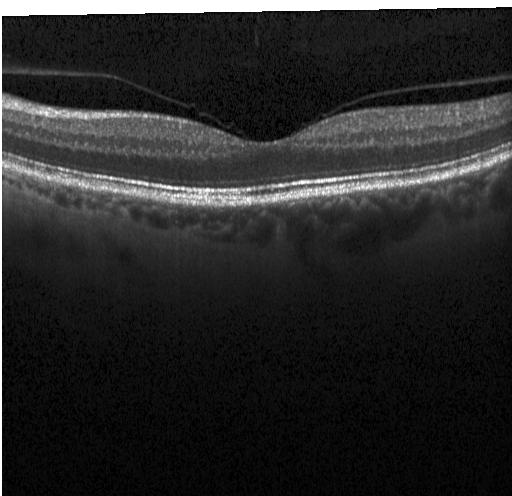 Retinal OCT B-scan; spectral-domain optical coherence tomography; acquired on a Heidelberg Spectralis
Finding: no evidence of CNV, DME, or drusen.